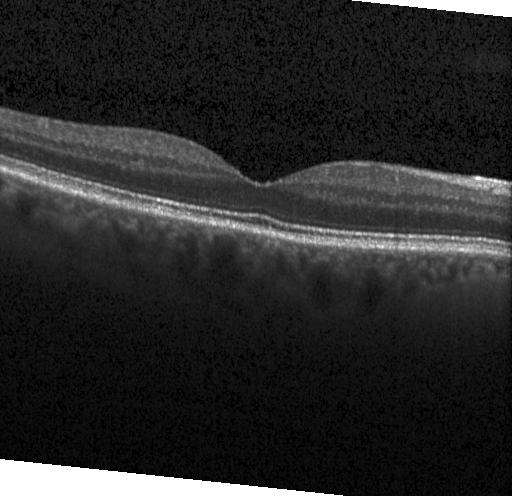 Heidelberg Spectralis. Optical coherence tomography scan
Neither choroidal neovascularization, diabetic macular edema, nor drusen.